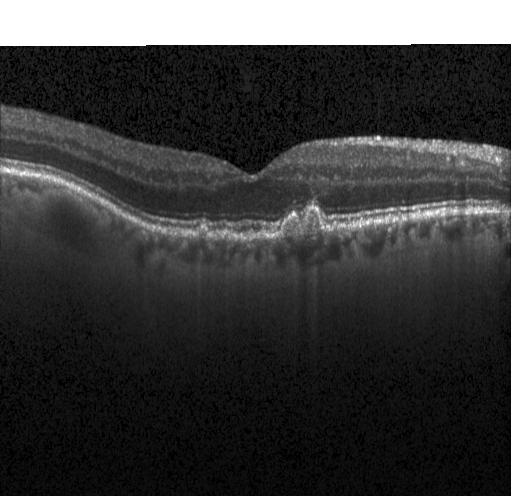
Finding: sub-RPE drusenoid deposits.